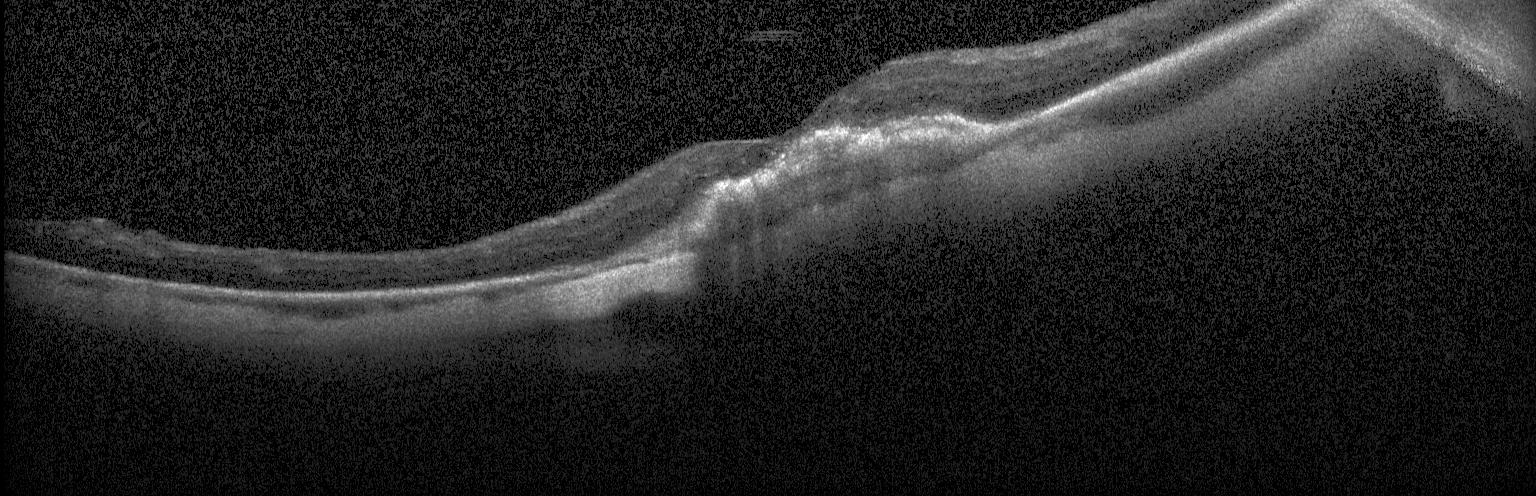
Optical coherence tomography scan. Spectral-domain OCT. Diagnosis: choroidal neovascularization (CNV).